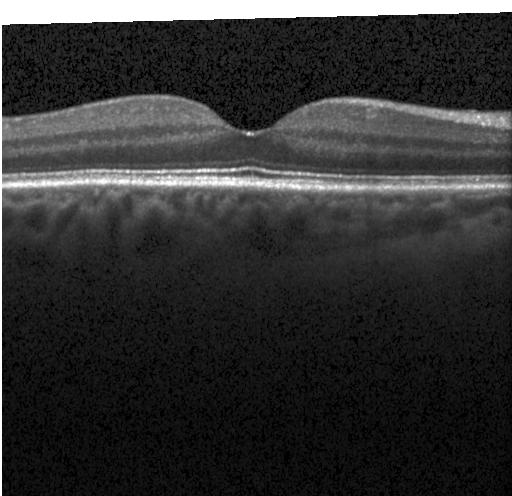
OCT scan showing no evidence of CNV, DME, or drusen.